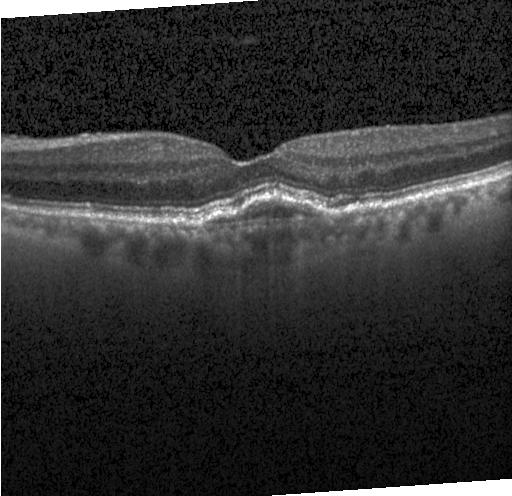
OCT B-scan
Macular OCT: CNV.